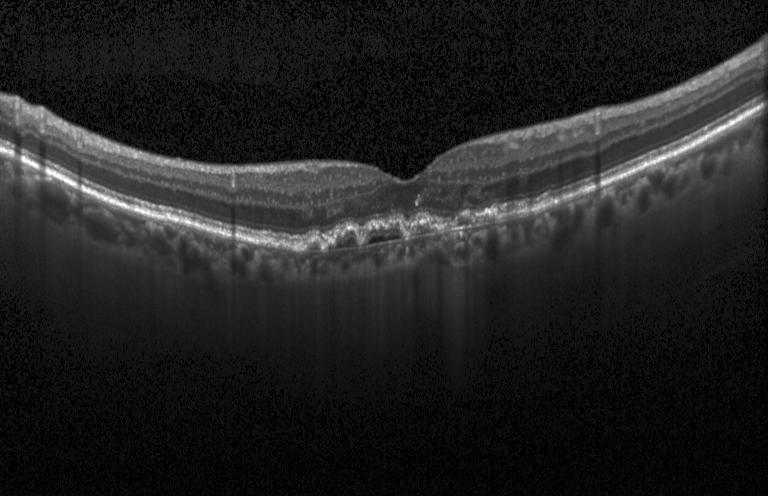 Acquired on a Heidelberg Spectralis · OCT line scan · spectral-domain OCT. Finding: a choroidal neovascular membrane.